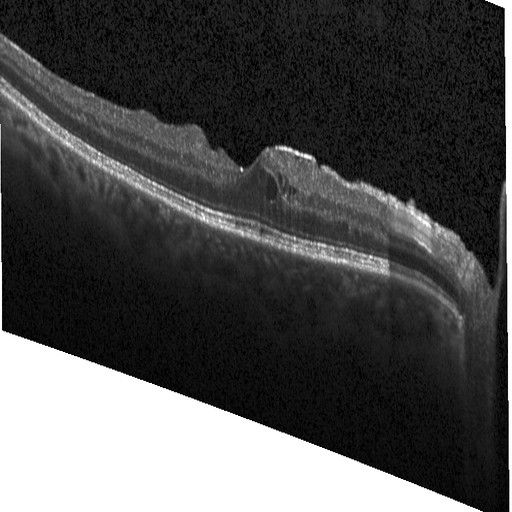 Impression: DME.